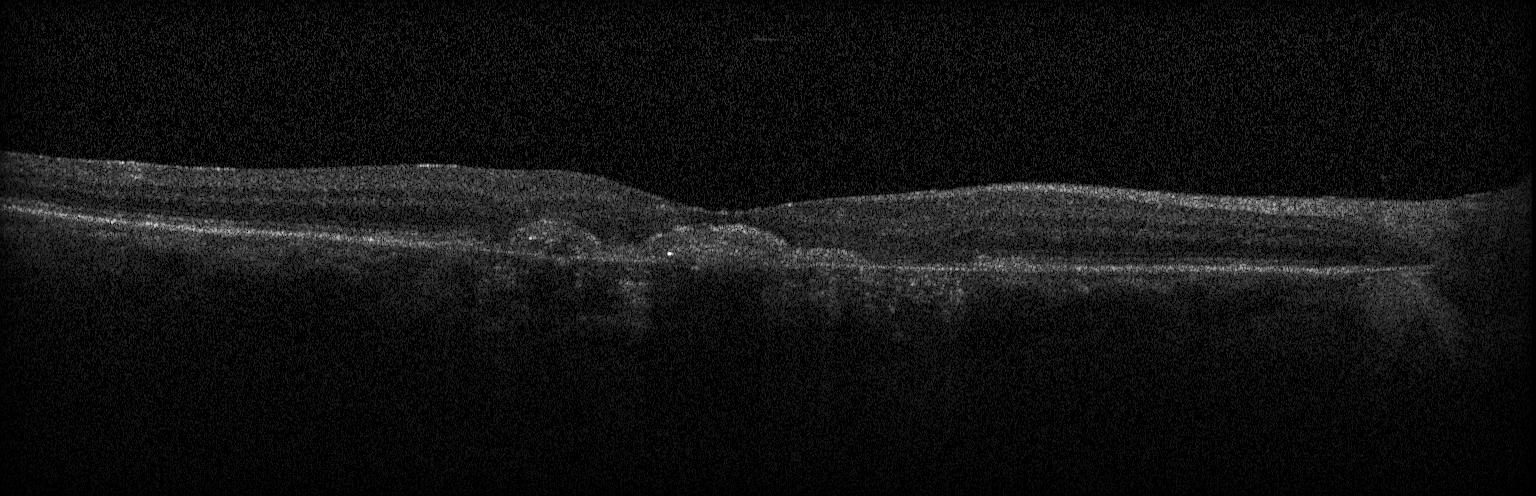
Diagnosis: a choroidal neovascular membrane.